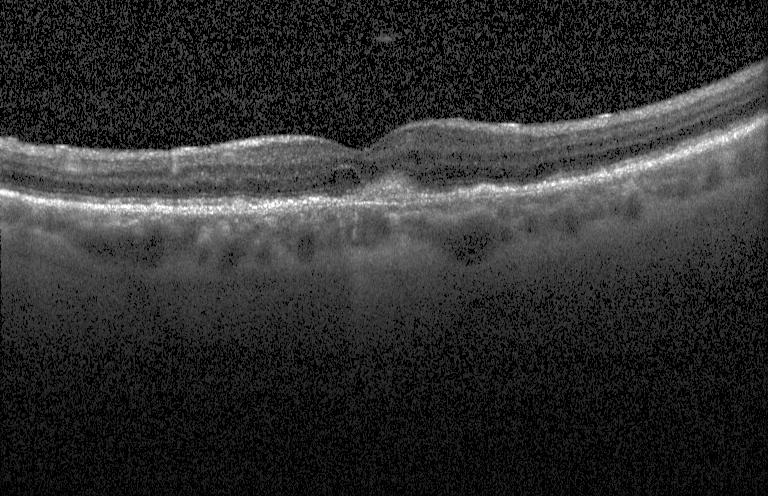
Finding: choroidal neovascularization (CNV).